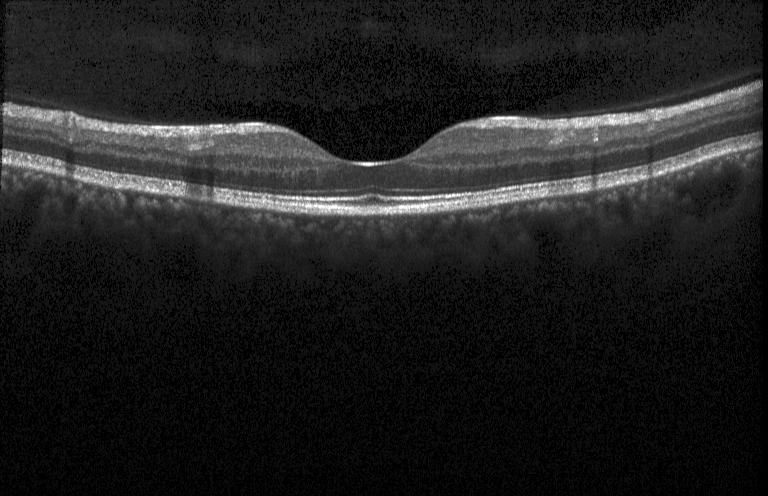

Spectral-domain OCT B-scan: no evidence of choroidal neovascularization, diabetic macular edema, or drusen.